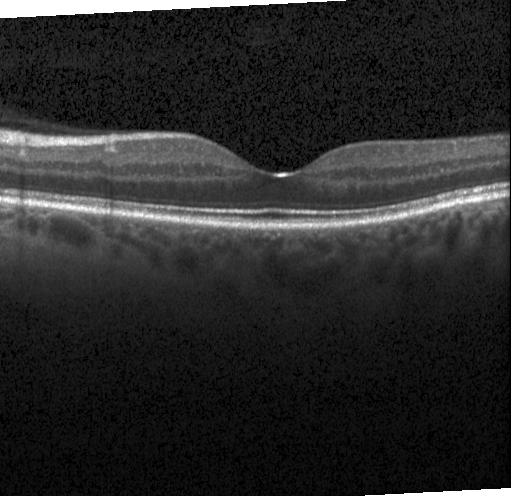

Spectral-domain optical coherence tomography; OCT line scan; macular scan.
This B-scan demonstrates no choroidal neovascularization, diabetic macular edema, or drusen.